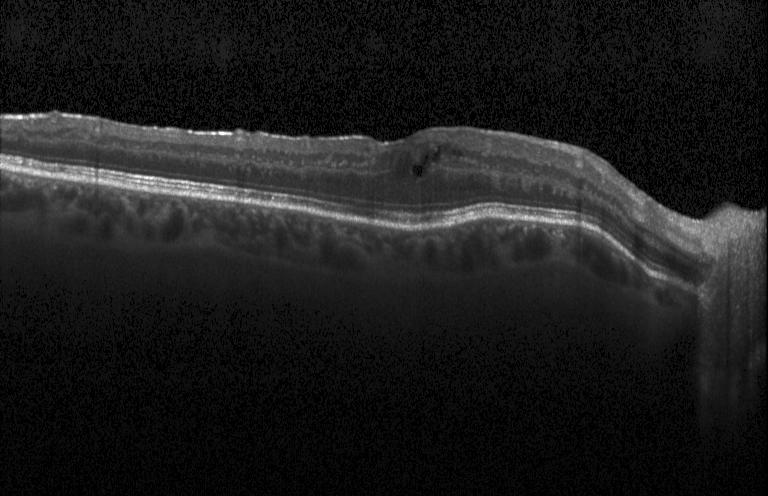 Spectral-domain OCT B-scan: diabetic macular edema.